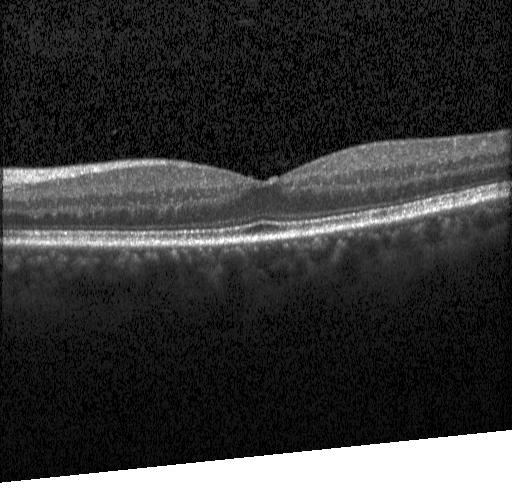 Diagnosis: neither CNV, DME, nor drusen.